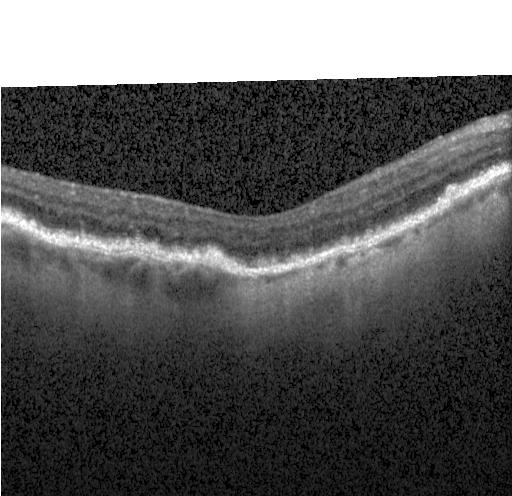
Spectral-domain OCT; OCT B-scan — CNV.